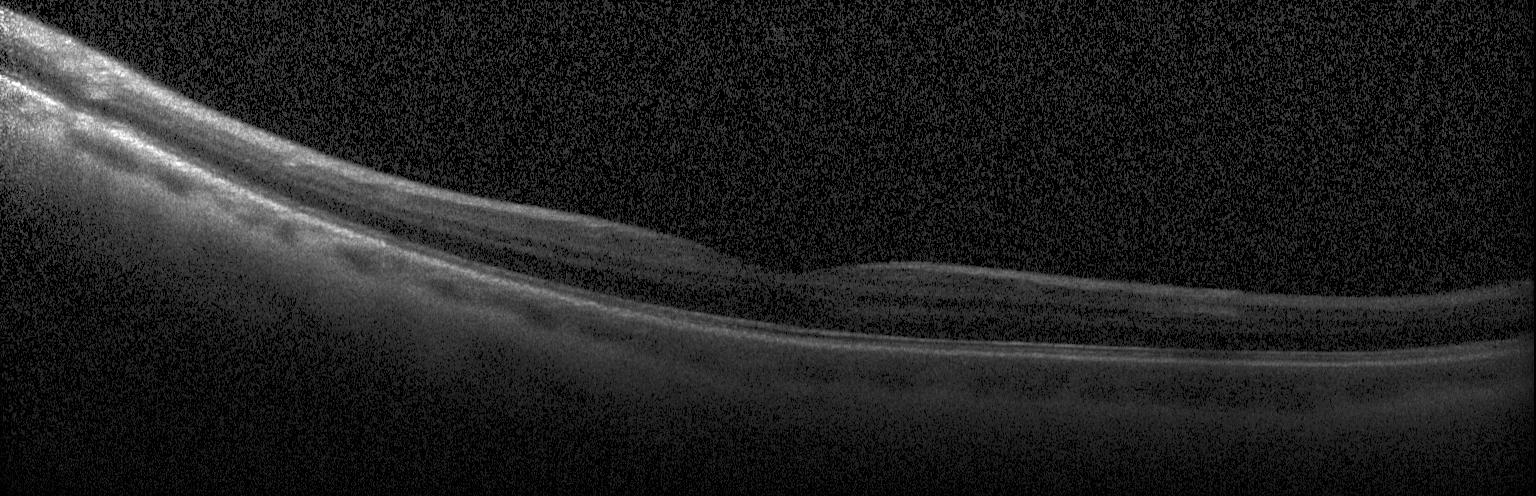
Optical coherence tomography B-scan
This B-scan demonstrates no choroidal neovascularization, diabetic macular edema, or drusen.